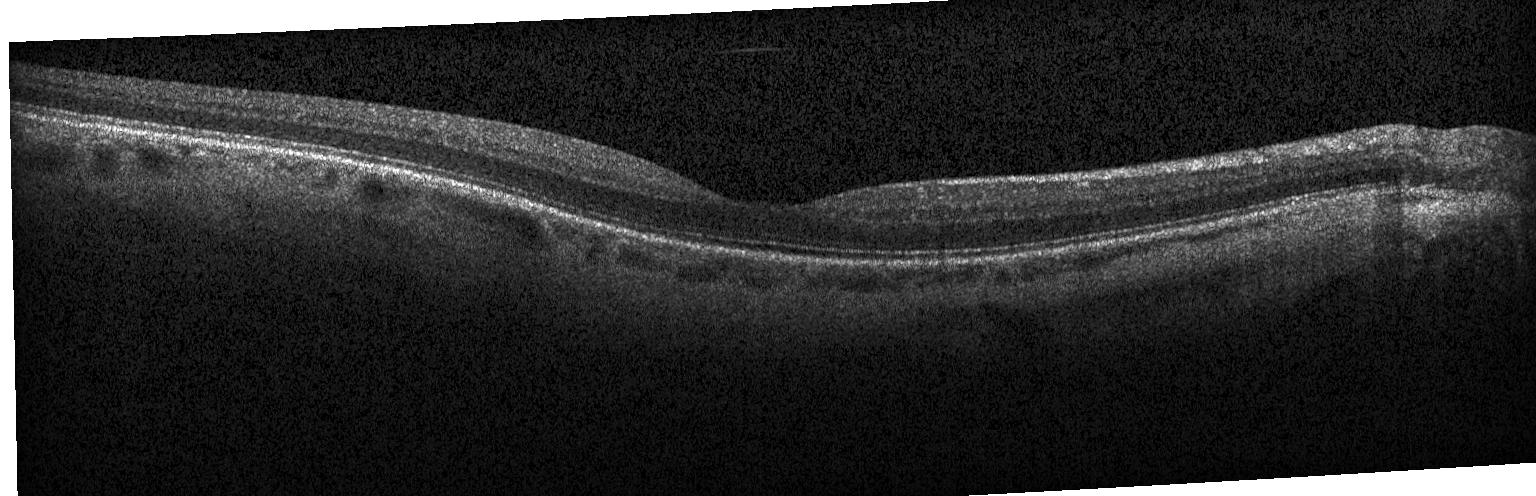
Macular OCT: no evidence of choroidal neovascularization, diabetic macular edema, or drusen.